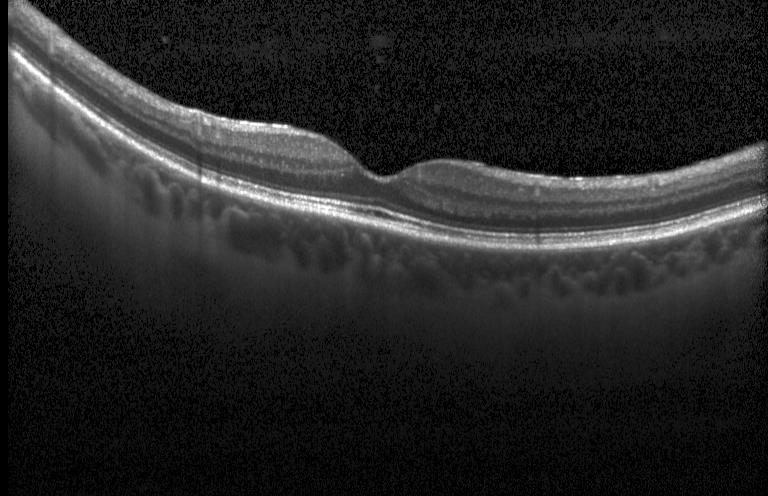 Impression: no evidence of choroidal neovascularization, diabetic macular edema, or drusen.